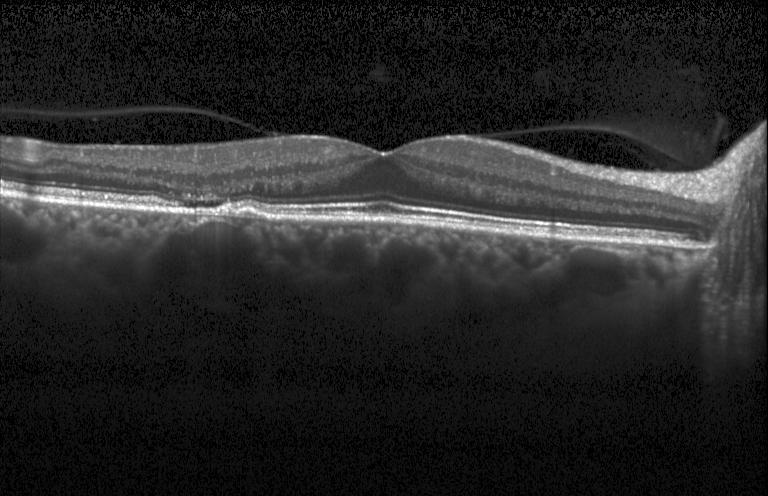
Heidelberg Spectralis OCT system · optical coherence tomography B-scan · through the macula · spectral-domain optical coherence tomography
Impression: a choroidal neovascular membrane.